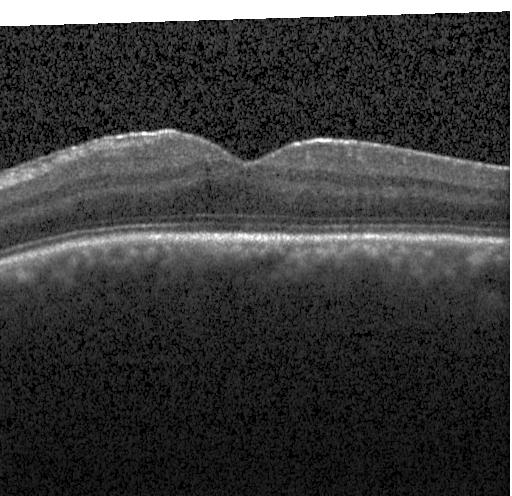 Through the macula. SD-OCT. Retinal OCT cross-section. Heidelberg Spectralis — Impression: no CNV, DME, or drusen.